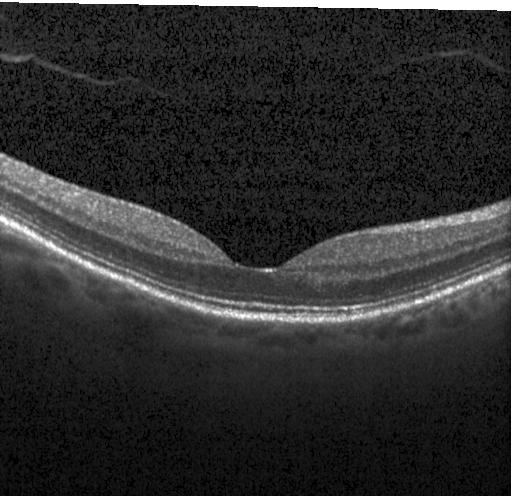 OCT finding: no CNV, no DME, and no drusen.